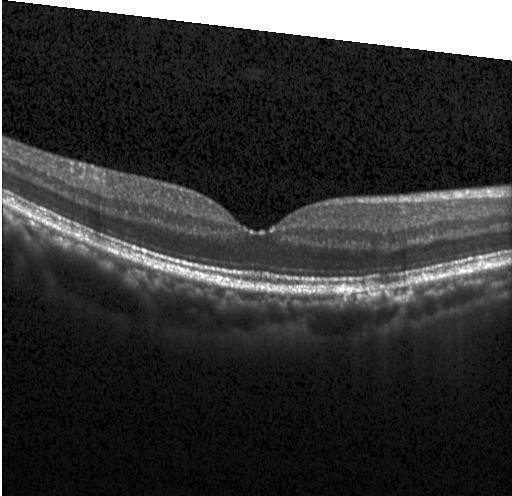
Acquired on a Heidelberg Spectralis, retinal OCT cross-section. Finding: no choroidal neovascularization, diabetic macular edema, or drusen.